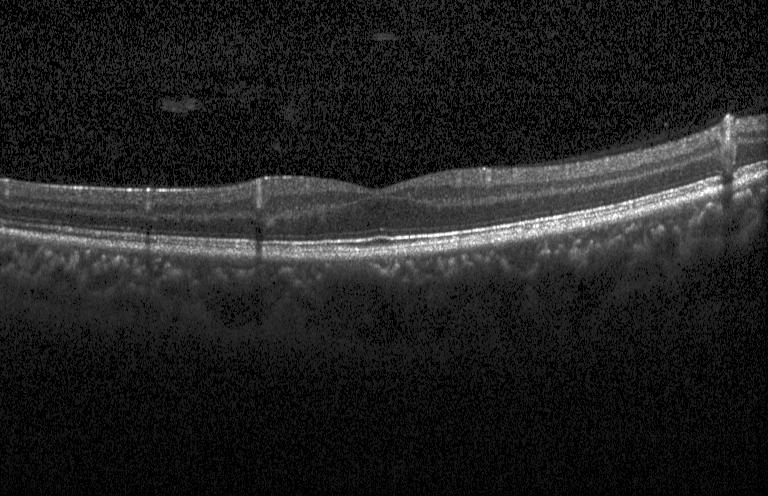 Optical coherence tomography B-scan, through the macula, acquired on a Heidelberg Spectralis, SD-OCT. OCT finding: no CNV, DME, or drusen.